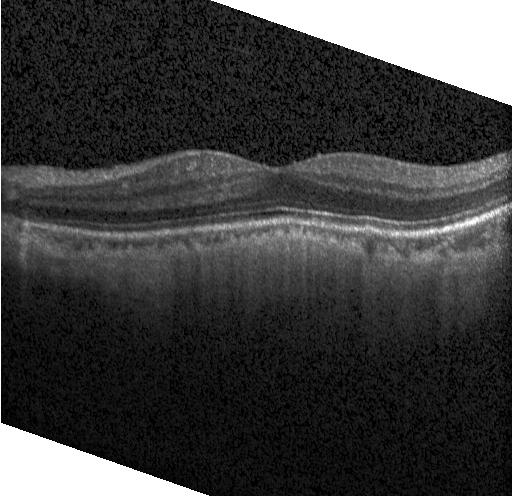

Diagnosis: no choroidal neovascularization, no diabetic macular edema, and no drusen.